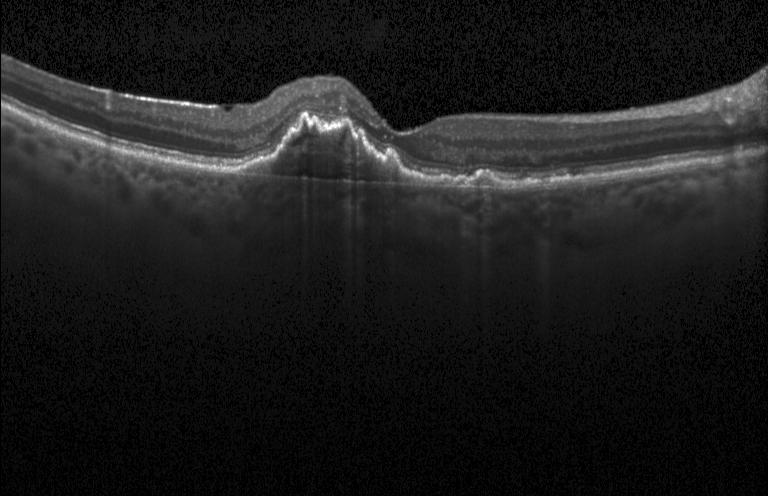

Assessment: a choroidal neovascular membrane.